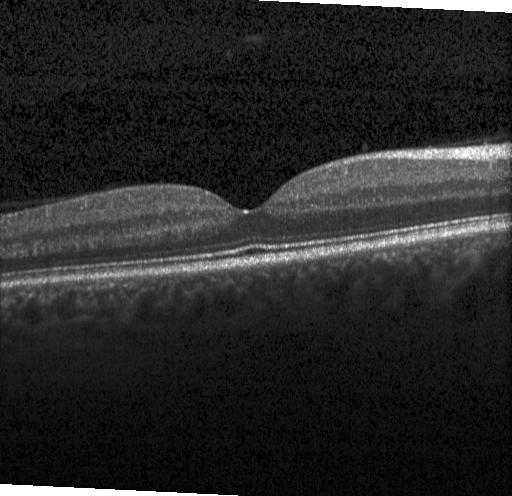
Dx: neither choroidal neovascularization, diabetic macular edema, nor drusen.